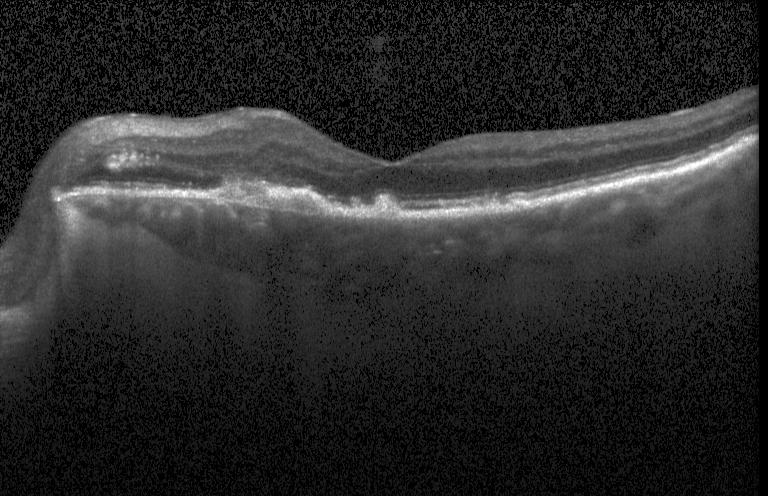
Horizontal scan through the fovea. OCT B-scan. Heidelberg Spectralis. SD-OCT
Macular OCT: choroidal neovascularization (CNV).